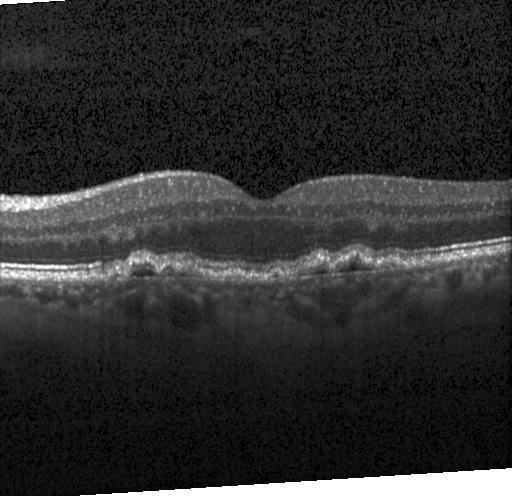
Optical coherence tomography scan; centered on the fovea; acquired on a Heidelberg Spectralis.
Impression: multiple drusen.